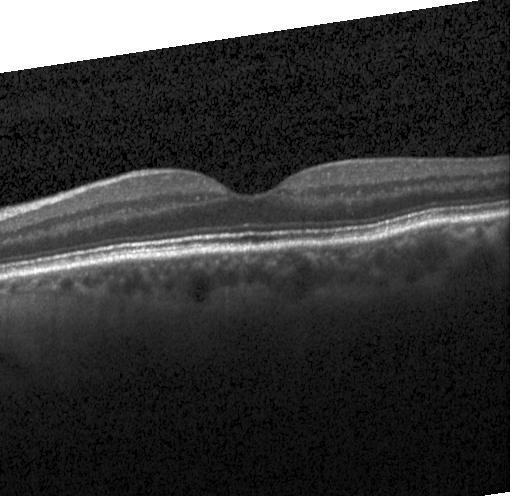 Instrument: Heidelberg Spectralis; optical coherence tomography B-scan; through the macula; SD-OCT — No evidence of choroidal neovascularization, diabetic macular edema, or drusen.